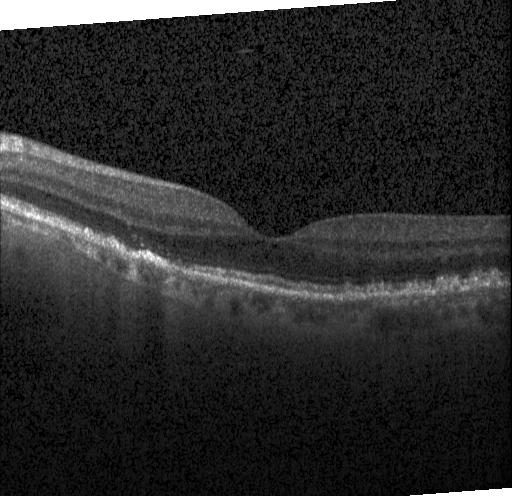 Horizontal scan through the fovea, optical coherence tomography scan, Heidelberg Spectralis.
Impression: sub-RPE drusenoid deposits.